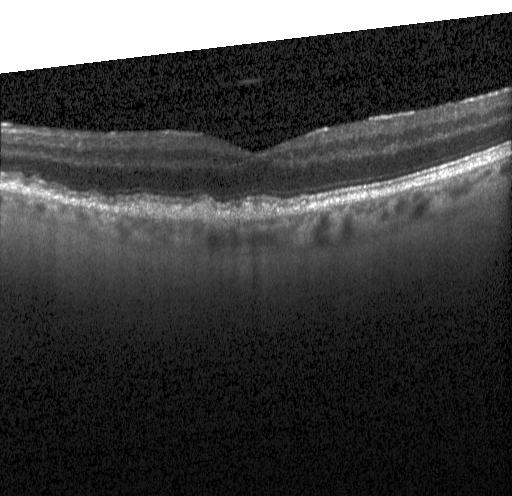

OCT finding: drusen.